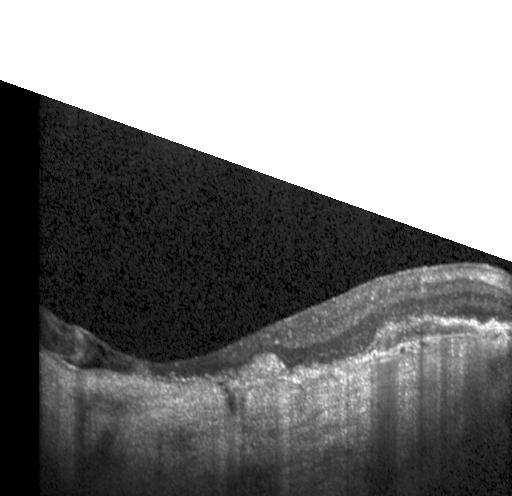 The scan shows a choroidal neovascular membrane.